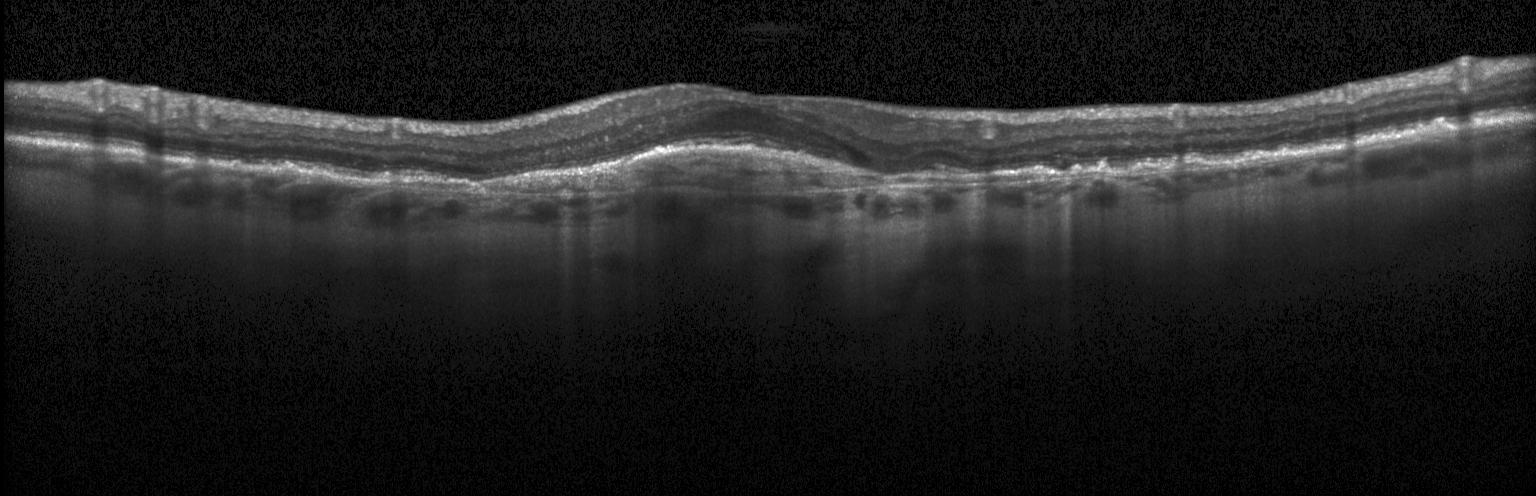

OCT scan showing a choroidal neovascular membrane.